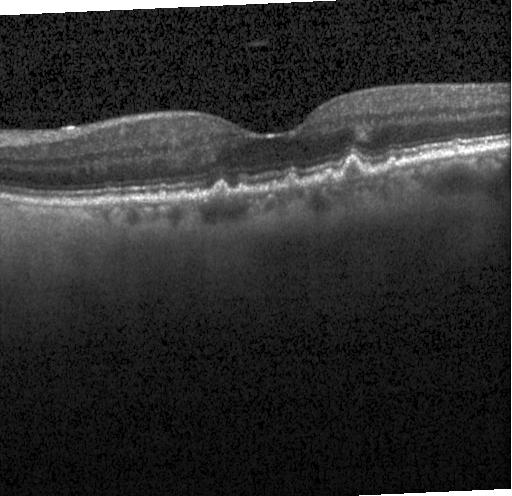
Heidelberg Spectralis. OCT line scan. Diagnosis: sub-RPE drusenoid deposits.